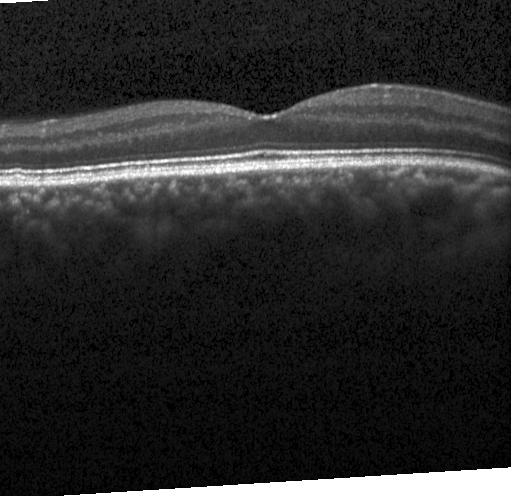 Spectral-domain optical coherence tomography. Fovea-centered. OCT line scan. Impression: neither choroidal neovascularization, diabetic macular edema, nor drusen.